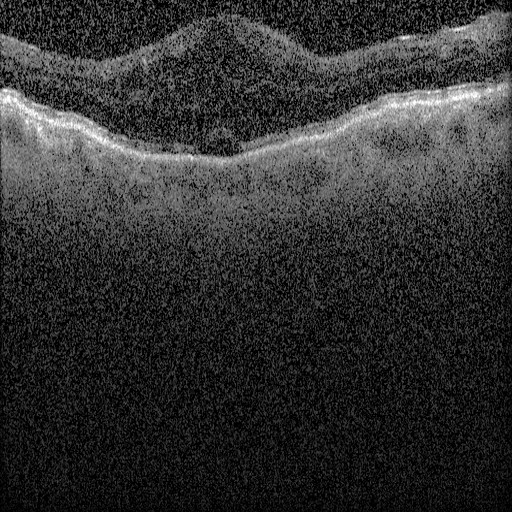
Retinal OCT cross-section; Heidelberg Spectralis; through the macula. Diagnosis: DME.